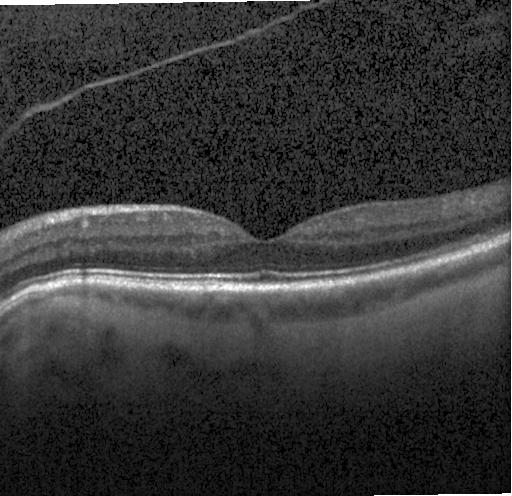
SD-OCT; acquired on a Heidelberg Spectralis; macular scan; optical coherence tomography scan — This B-scan demonstrates no evidence of choroidal neovascularization, diabetic macular edema, or drusen.